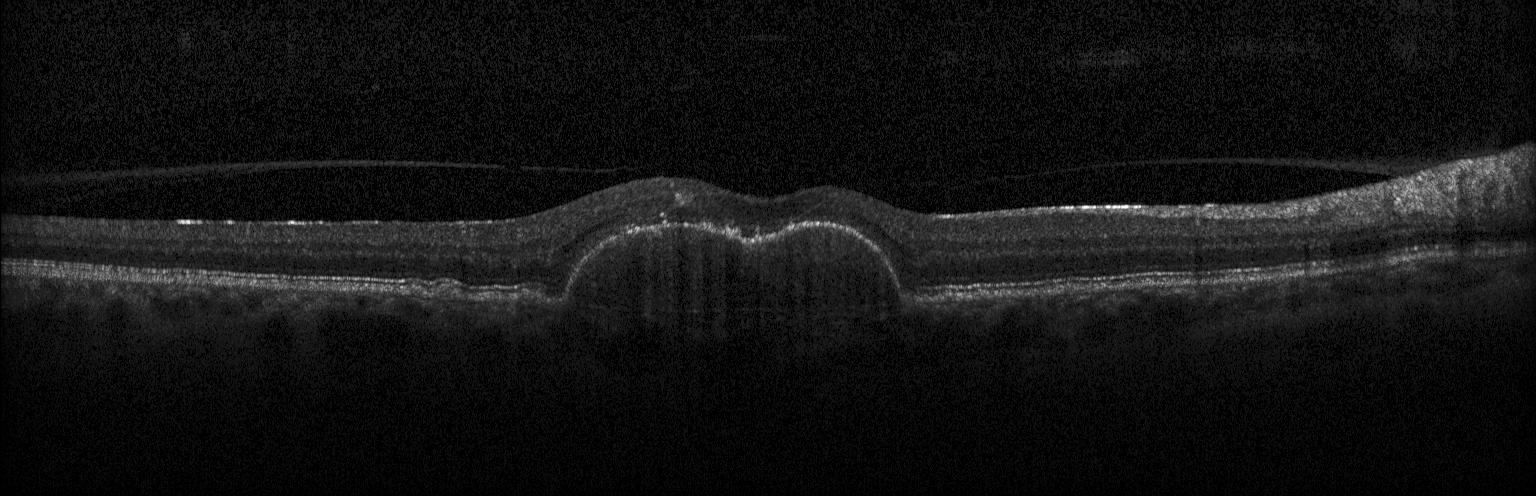
Macular scan; optical coherence tomography B-scan
Diagnosis: CNV.